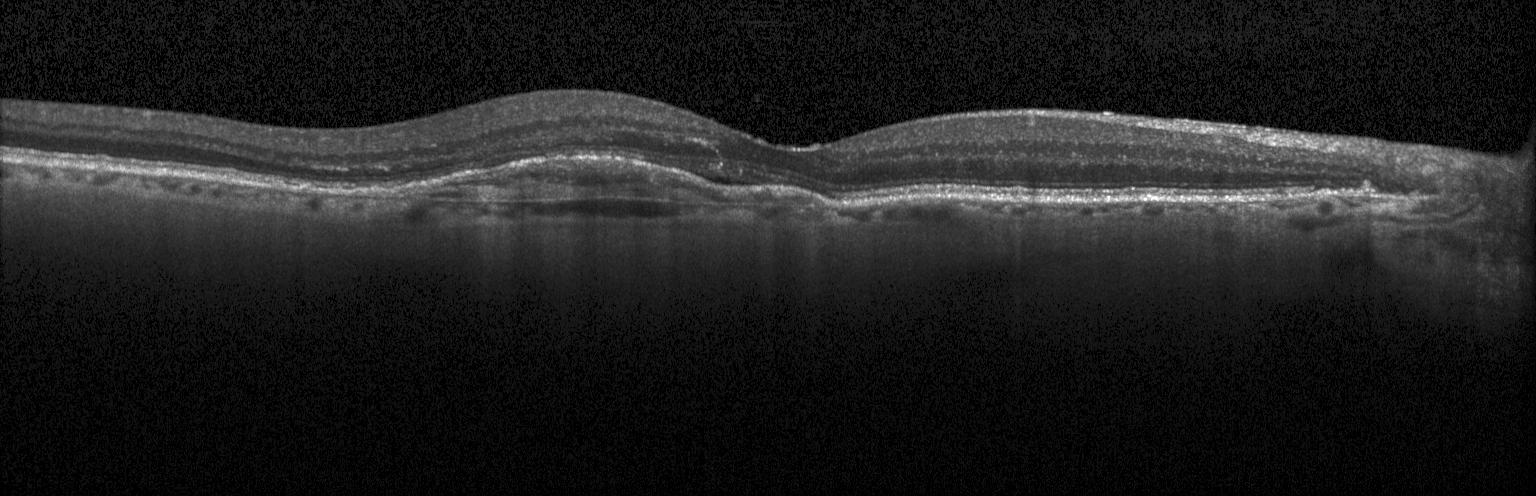

Optical coherence tomography scan. Instrument: Heidelberg Spectralis
Impression: a choroidal neovascular membrane.